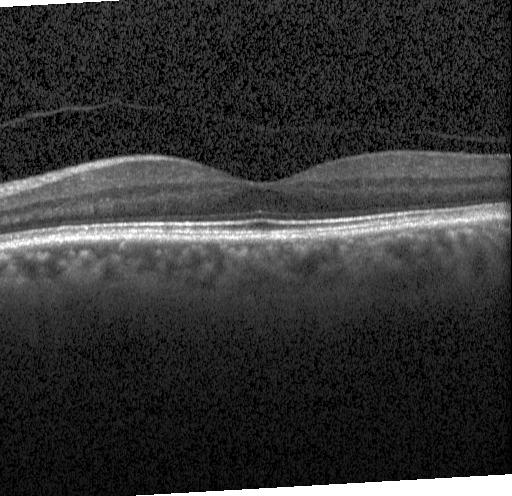

OCT scan showing no choroidal neovascularization, diabetic macular edema, or drusen.